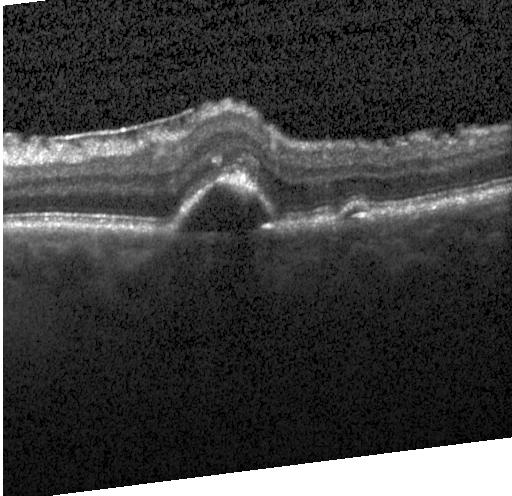 Finding: choroidal neovascularization.